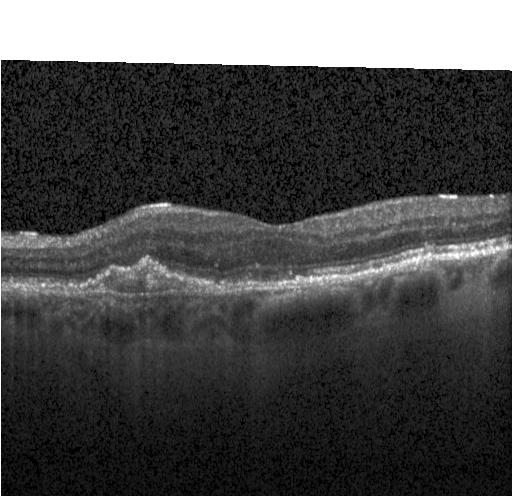 Macular OCT demonstrating choroidal neovascularization (CNV).